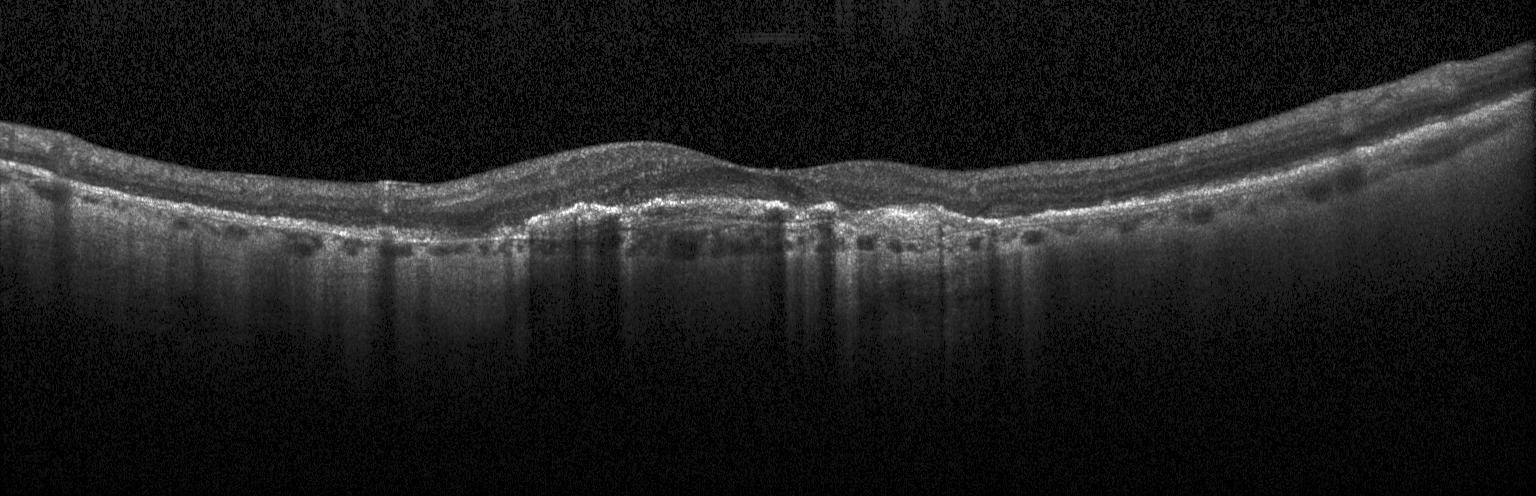
The scan shows choroidal neovascularization.